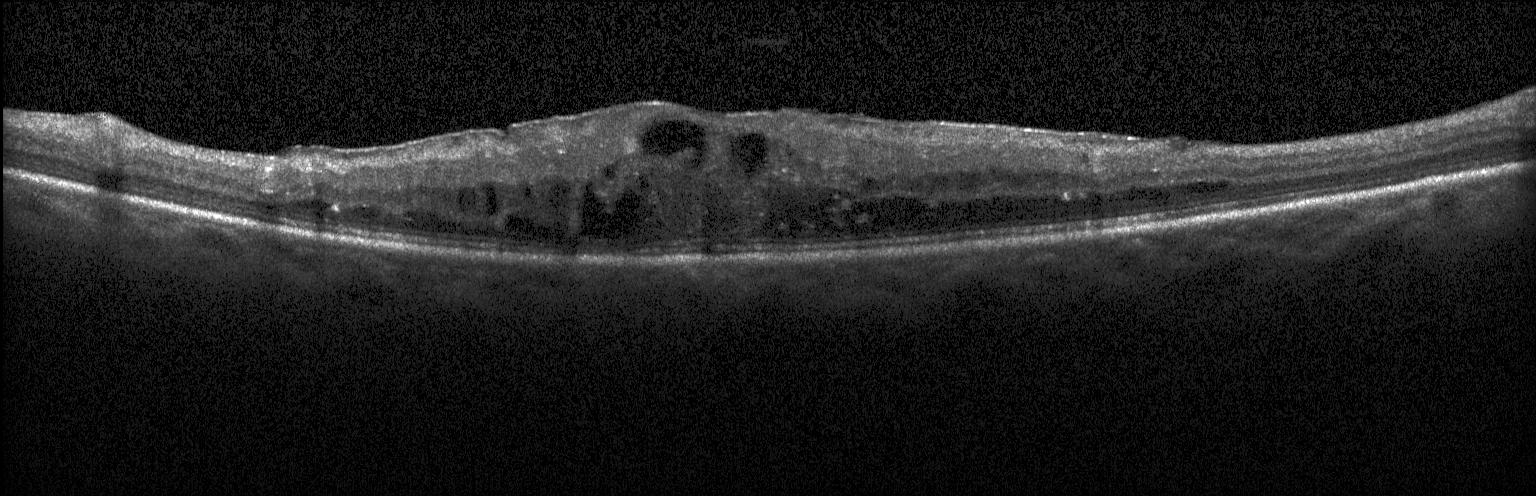

Instrument: Heidelberg Spectralis; optical coherence tomography scan; spectral-domain optical coherence tomography.
Impression: diabetic macular edema.